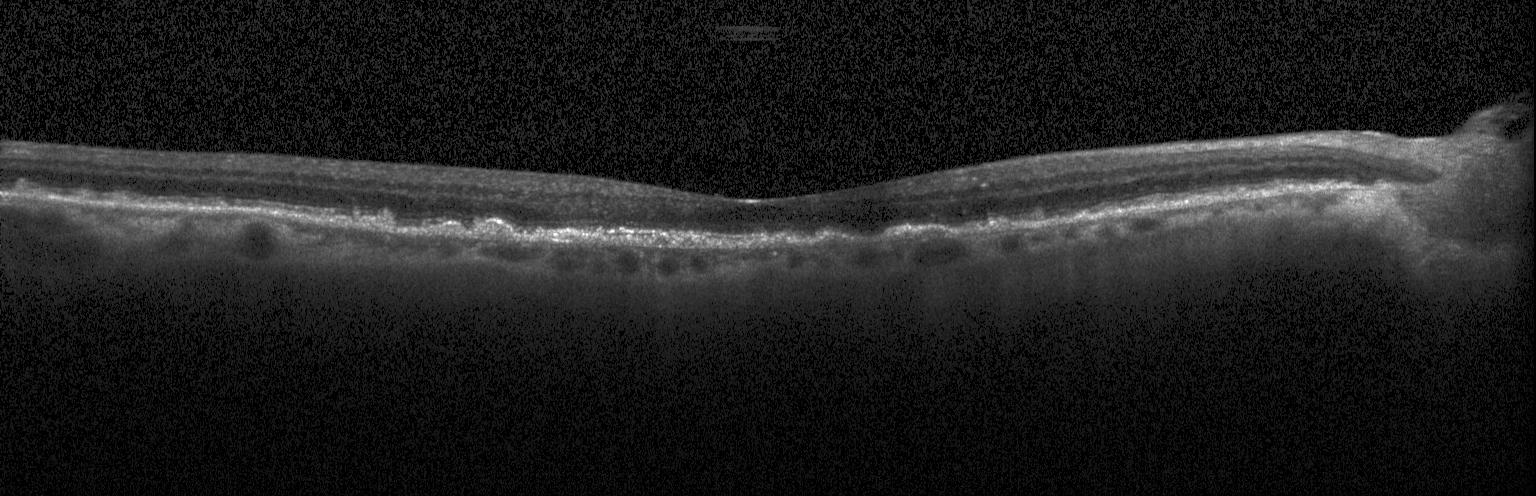
Diagnosis: a choroidal neovascular membrane.